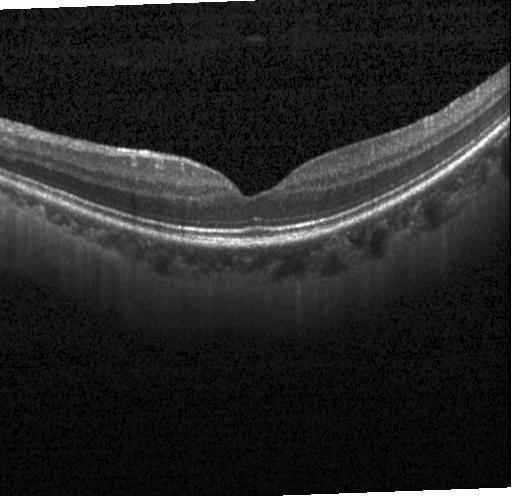

Horizontal scan through the fovea; retinal OCT cross-section; spectral-domain optical coherence tomography; Heidelberg Spectralis OCT system.
Impression: no choroidal neovascularization, diabetic macular edema, or drusen.